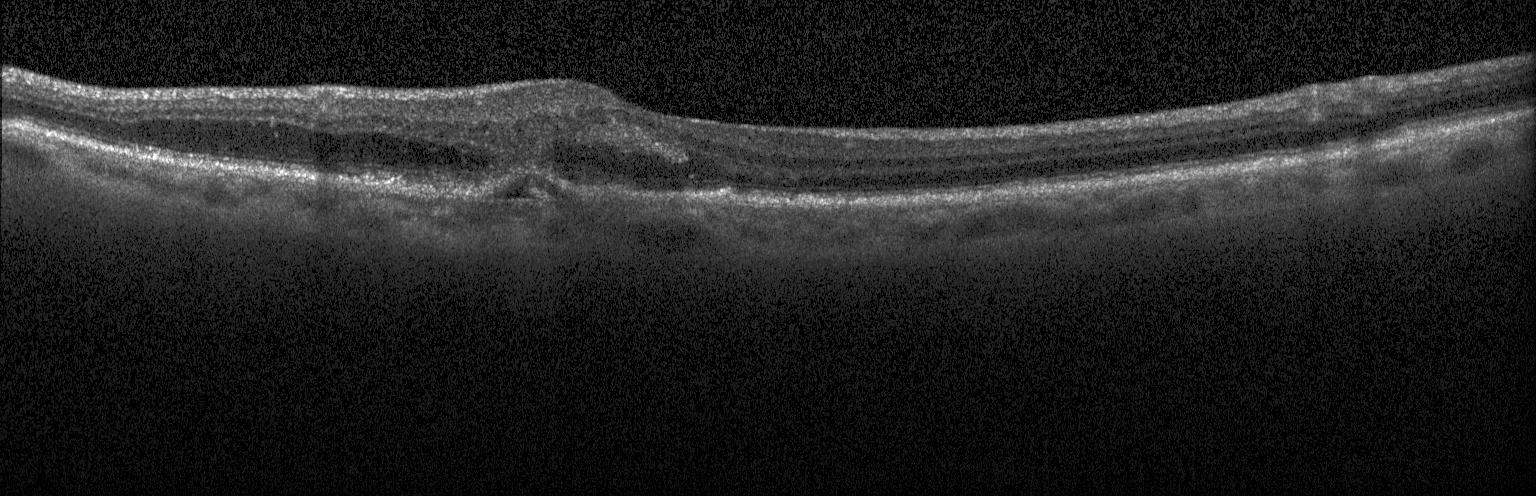

Retinal OCT B-scan
Diagnosis: a choroidal neovascular membrane.